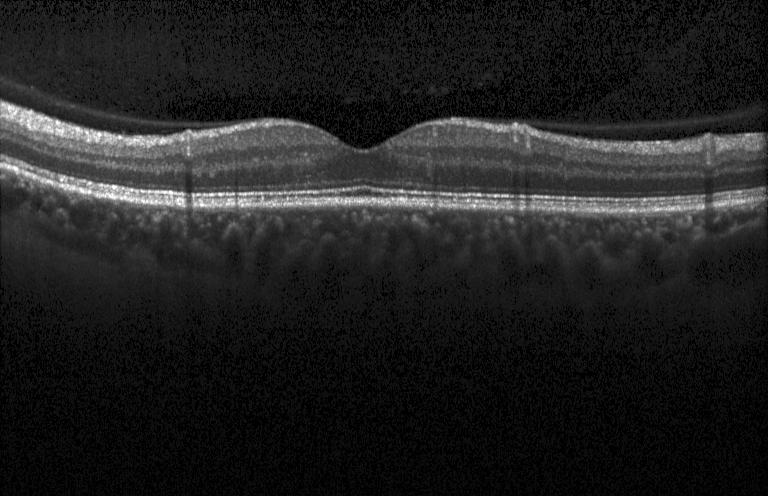

Impression: no choroidal neovascularization, diabetic macular edema, or drusen.